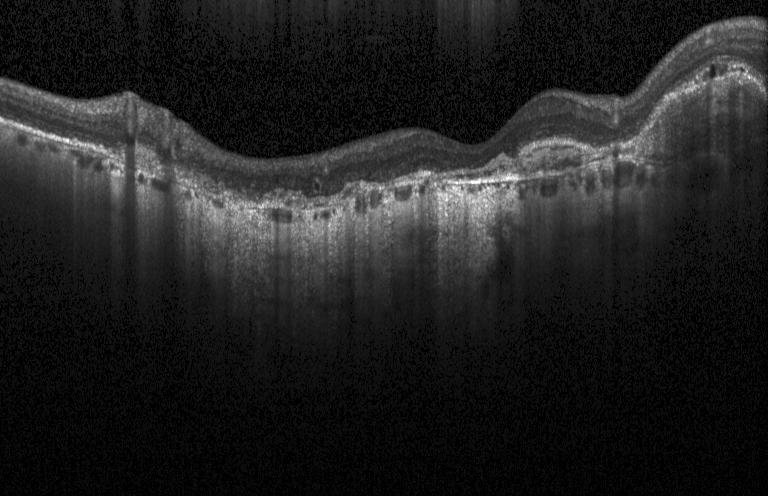

Retinal OCT B-scan — Diagnosis: a choroidal neovascular membrane.